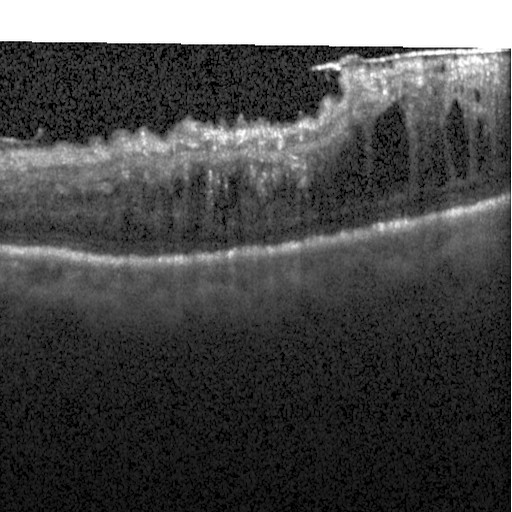

Dx: diabetic macular edema.